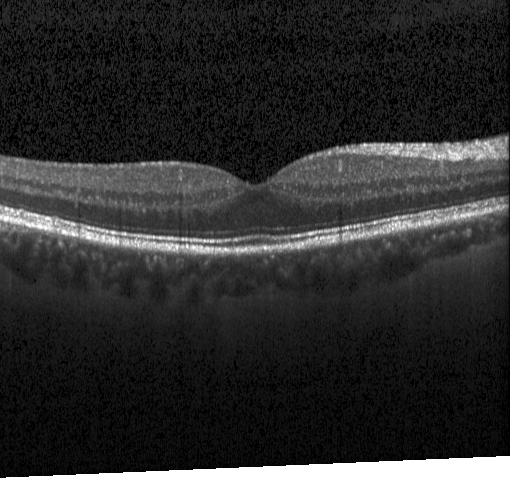 Optical coherence tomography scan. Heidelberg Spectralis OCT system
Assessment: no choroidal neovascularization, no diabetic macular edema, and no drusen.